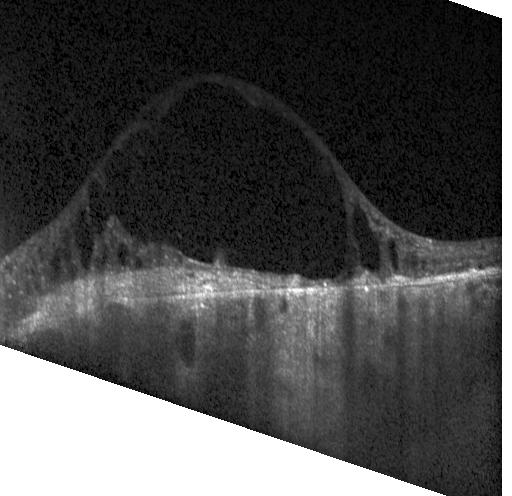
Centered on the fovea. SD-OCT. Optical coherence tomography B-scan. This B-scan demonstrates choroidal neovascularization.